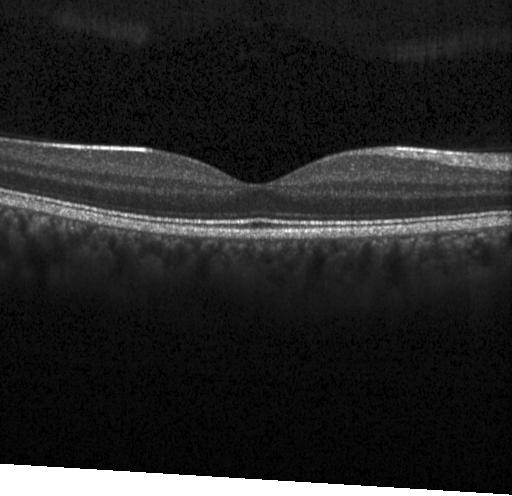

The scan shows neither CNV, DME, nor drusen.